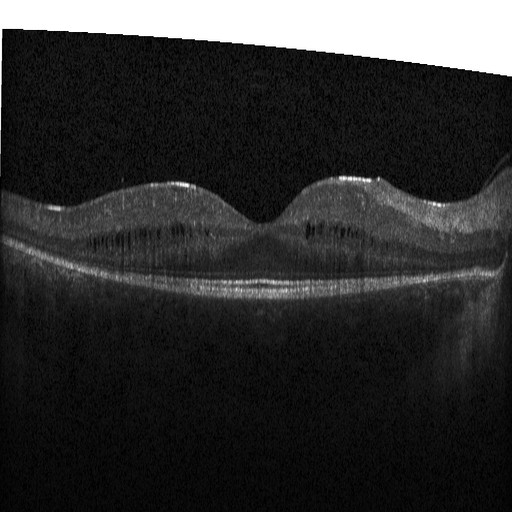 Macular scan. Spectral-domain OCT. Instrument: Heidelberg Spectralis. Retinal OCT cross-section — Impression: DME.